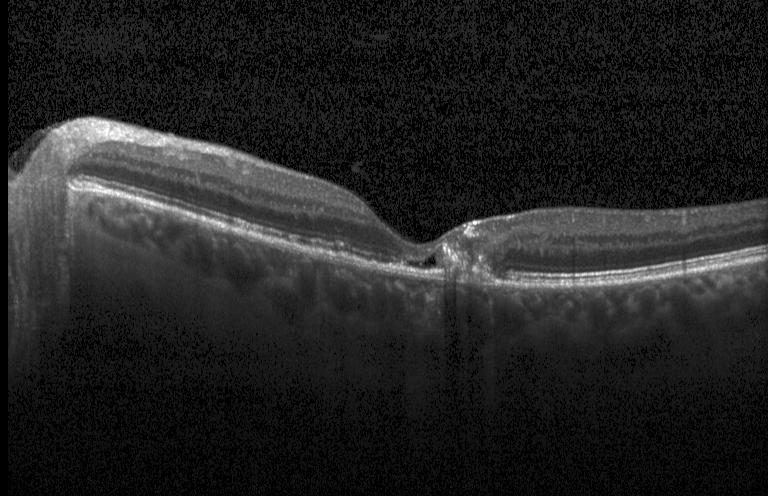 OCT line scan · instrument: Heidelberg Spectralis. The scan shows choroidal neovascularization (CNV).